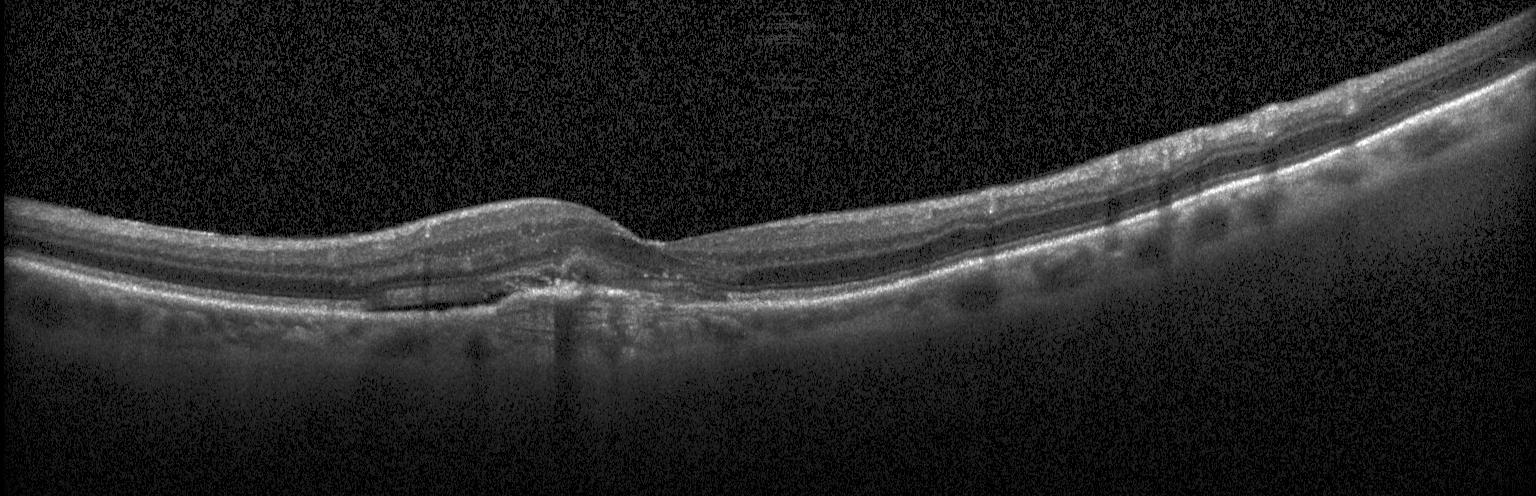
Optical coherence tomography scan. Finding: a choroidal neovascular membrane.